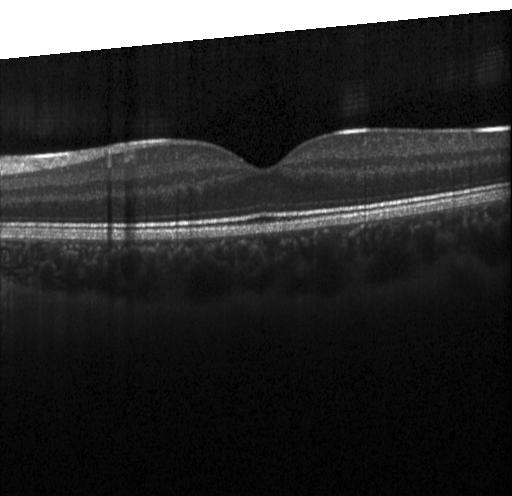 Optical coherence tomography scan; spectral-domain optical coherence tomography
OCT finding: no CNV, DME, or drusen.